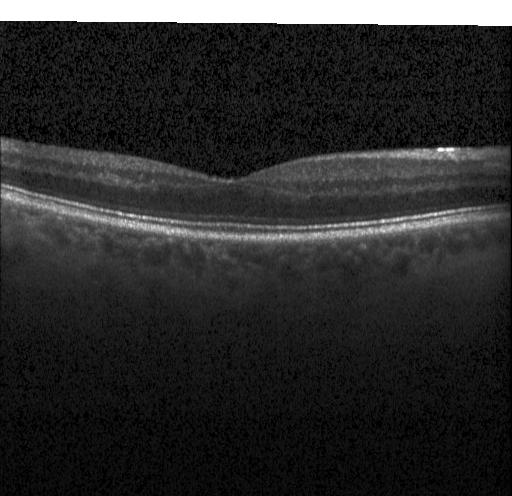

Macular OCT: no choroidal neovascularization, no diabetic macular edema, and no drusen.